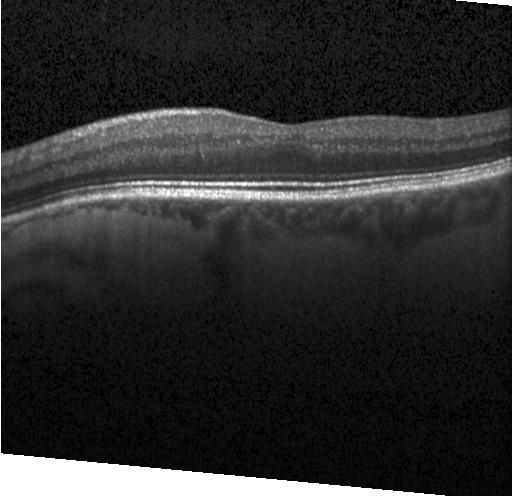 Diagnosis: no evidence of choroidal neovascularization, diabetic macular edema, or drusen.